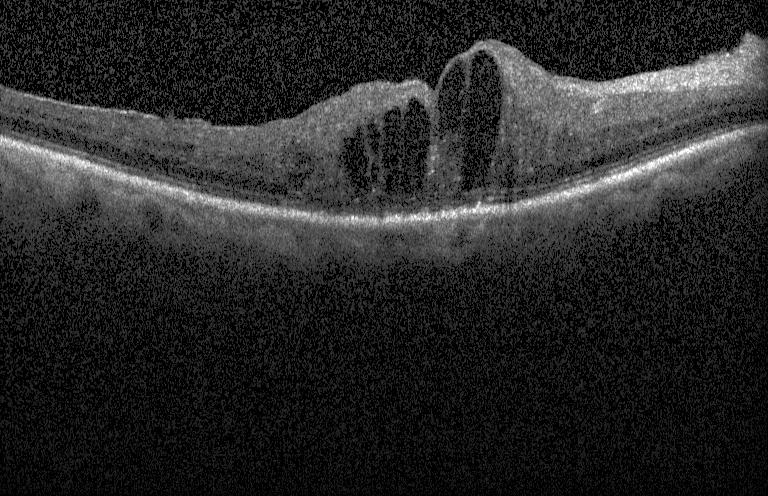

Through the macula. Retinal OCT B-scan. Instrument: Heidelberg Spectralis
The scan shows diabetic macular edema (DME).